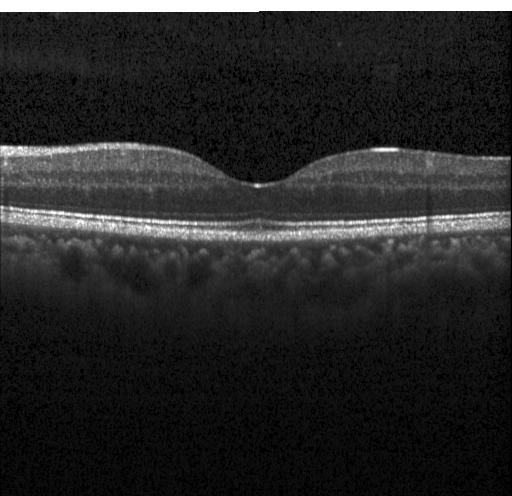
Acquired on a Heidelberg Spectralis. Retinal OCT cross-section. Diagnosis: no CNV, no DME, and no drusen.